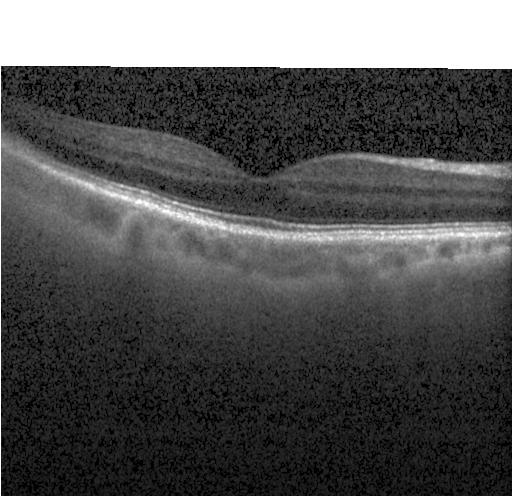

Dx: no CNV, DME, or drusen.